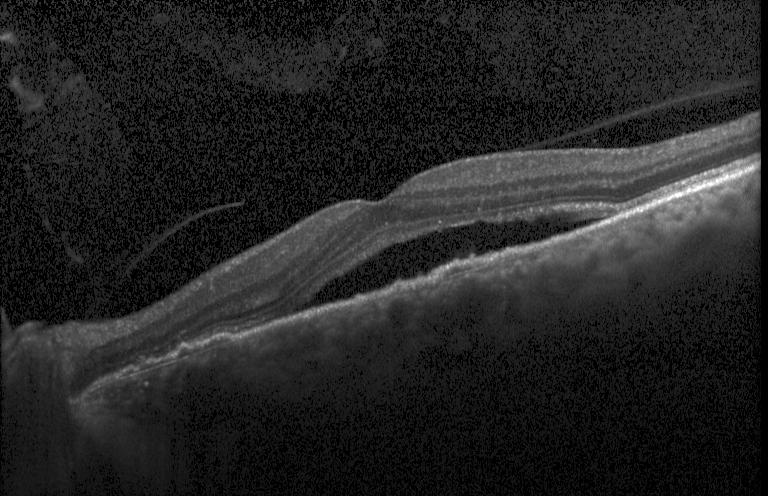

Retinal OCT cross-section
OCT finding: choroidal neovascularization (CNV).